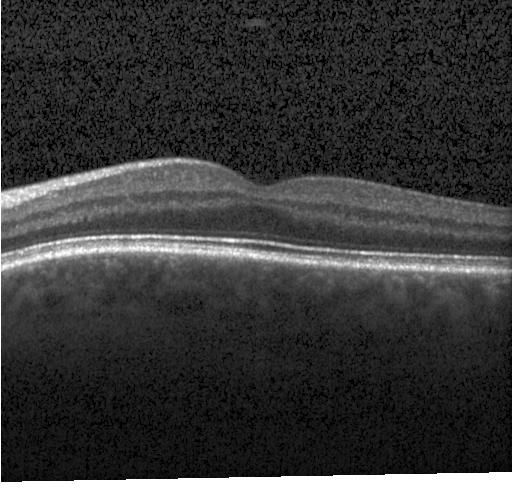 SD-OCT, retinal OCT B-scan, Heidelberg Spectralis. Assessment: no CNV, DME, or drusen.